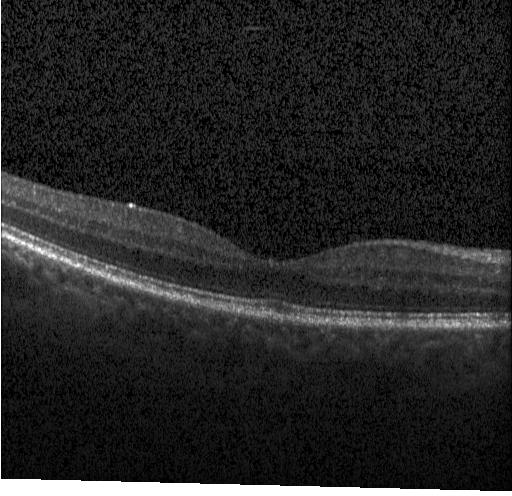
Optical coherence tomography B-scan, horizontal scan through the fovea.
No choroidal neovascularization, no diabetic macular edema, and no drusen.